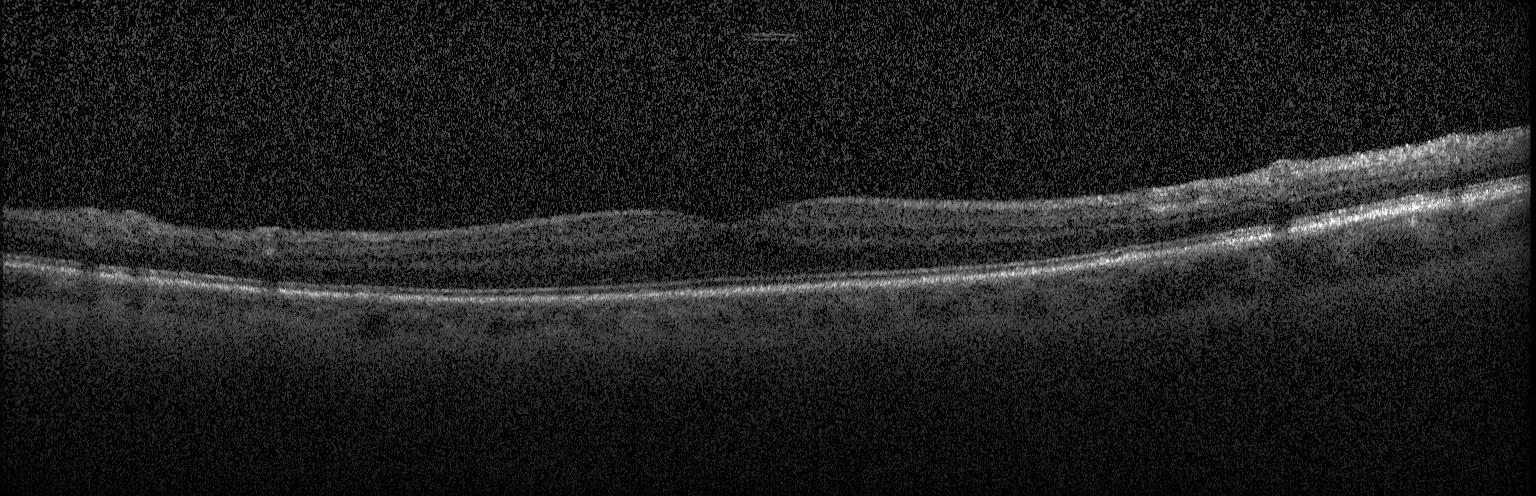
Optical coherence tomography scan; SD-OCT; acquired on a Heidelberg Spectralis; through the macula.
No evidence of choroidal neovascularization, diabetic macular edema, or drusen.